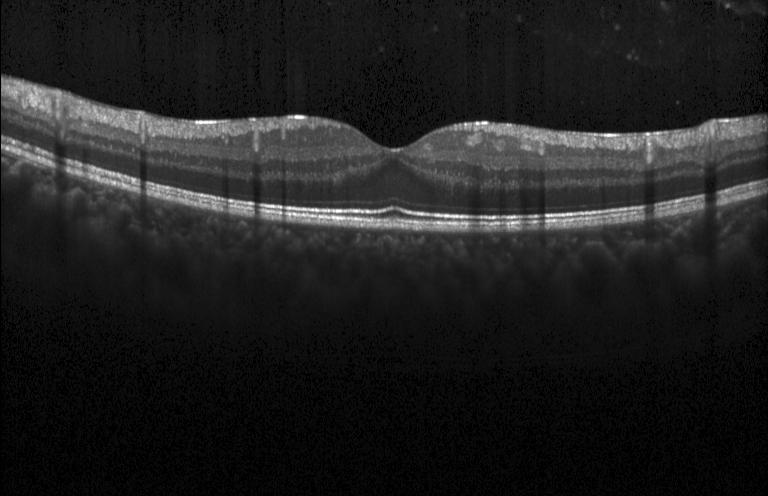

SD-OCT, Heidelberg Spectralis OCT system, macular scan, retinal OCT B-scan.
This B-scan demonstrates no evidence of choroidal neovascularization, diabetic macular edema, or drusen.